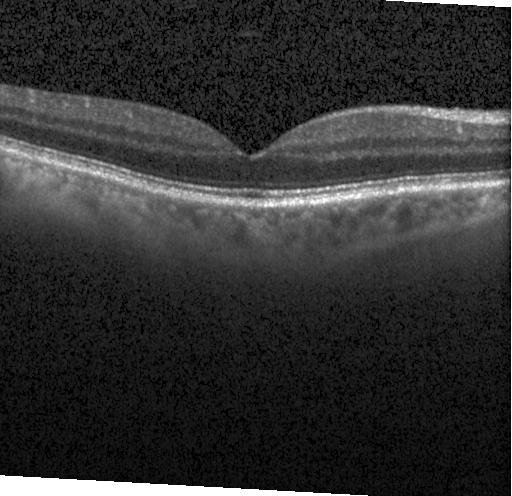 OCT line scan — OCT finding: no evidence of CNV, DME, or drusen.